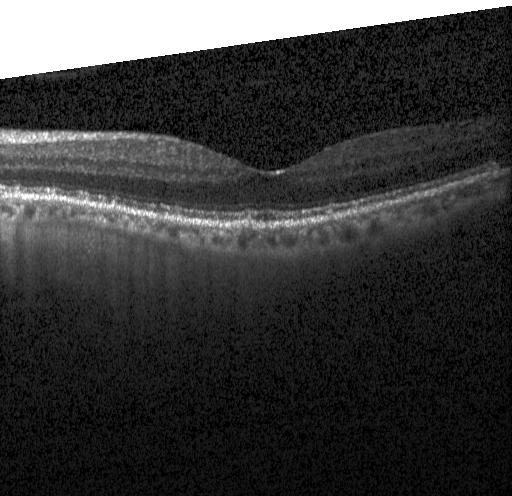
OCT B-scan; Heidelberg Spectralis OCT system; spectral-domain OCT. Dx: neither choroidal neovascularization, diabetic macular edema, nor drusen.